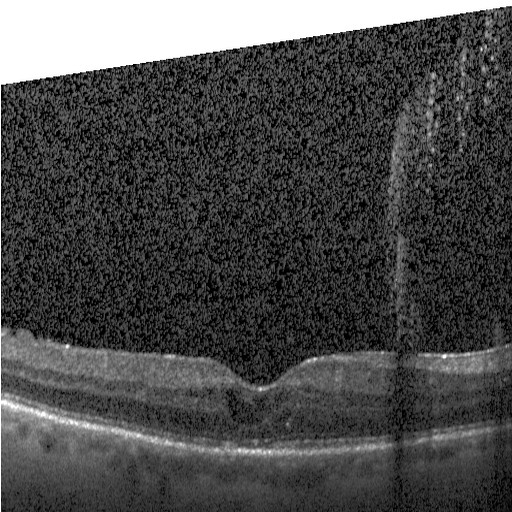

Retinal OCT cross-section. Diabetic macular edema.